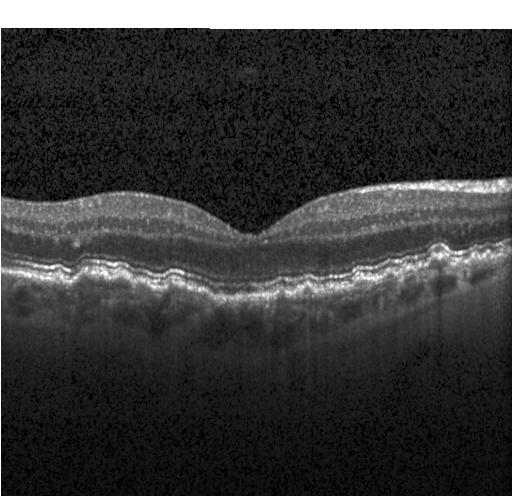 Retinal OCT B-scan
Impression: sub-RPE drusenoid deposits.